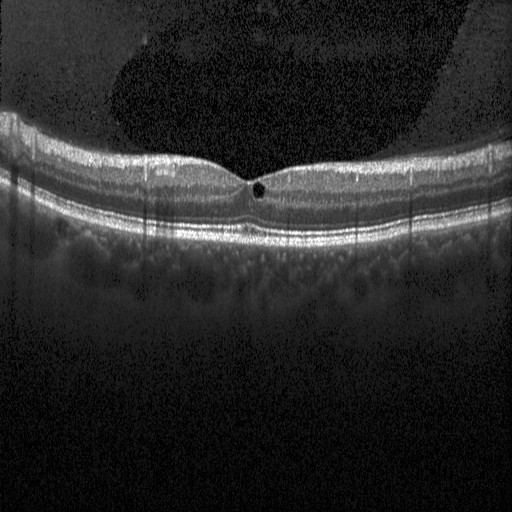
Macular scan. Spectral-domain optical coherence tomography. Heidelberg Spectralis. Retinal OCT cross-section. Impression: DME.